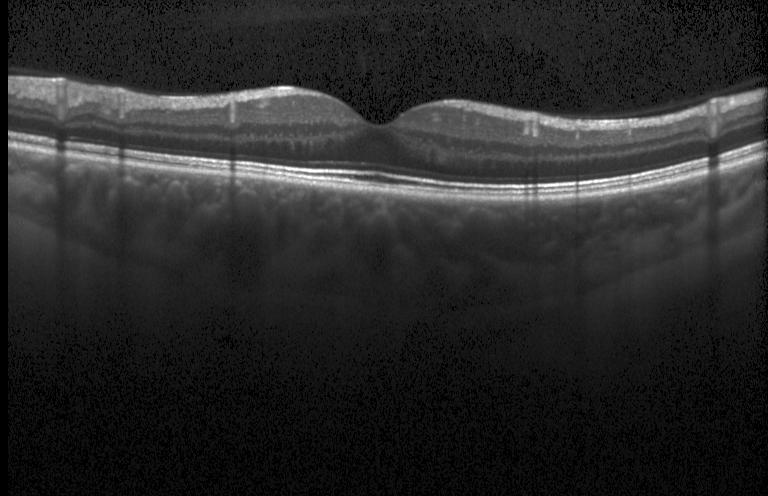

Optical coherence tomography scan — Finding: neither choroidal neovascularization, diabetic macular edema, nor drusen.